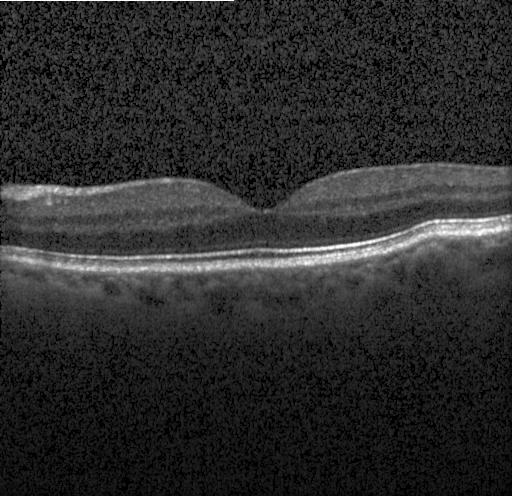
No evidence of choroidal neovascularization, diabetic macular edema, or drusen.